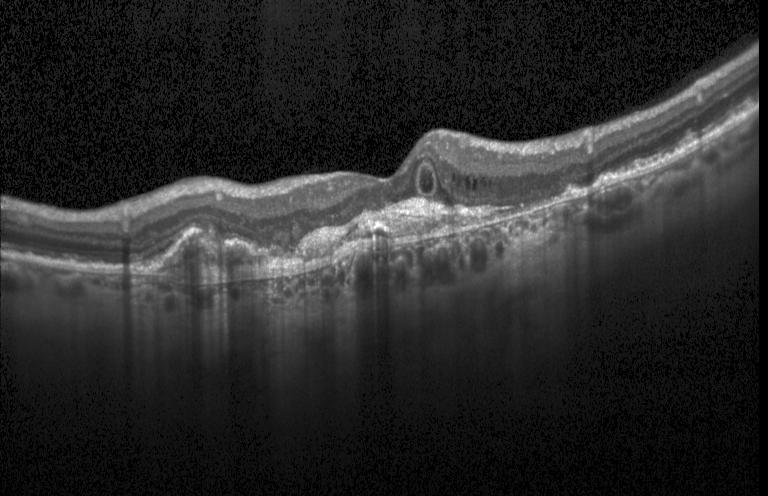 Retinal OCT cross-section.
Diagnosis: choroidal neovascularization (CNV).